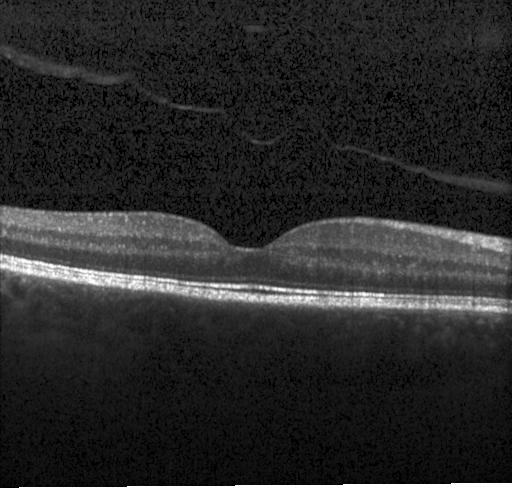

Heidelberg Spectralis, retinal OCT B-scan, spectral-domain optical coherence tomography, horizontal scan through the fovea
The scan shows neither choroidal neovascularization, diabetic macular edema, nor drusen.